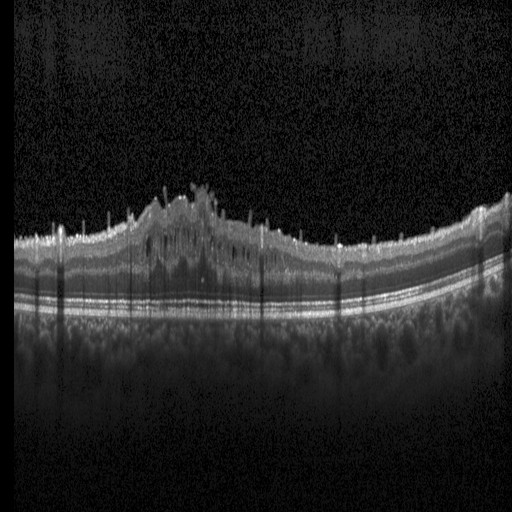
Centered on the fovea. Optical coherence tomography scan. SD-OCT. Acquired on a Heidelberg Spectralis — Dx: DME.